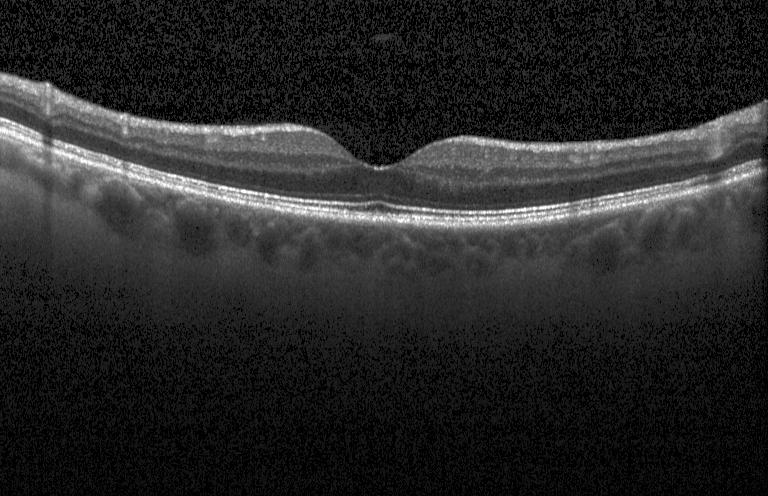
Macular OCT: no evidence of CNV, DME, or drusen.